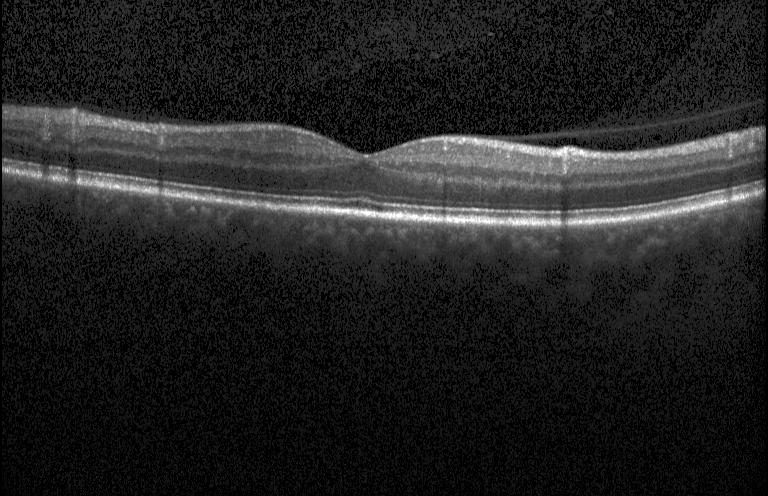

Finding: no choroidal neovascularization, diabetic macular edema, or drusen.